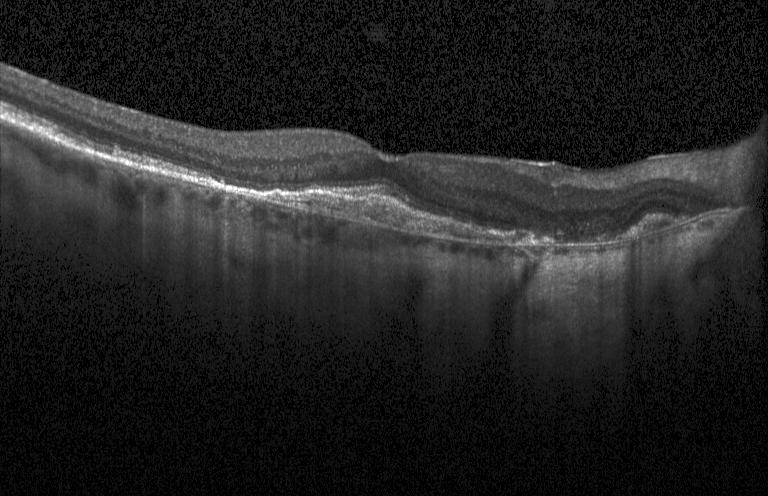

Spectral-domain optical coherence tomography, optical coherence tomography scan — The scan shows a choroidal neovascular membrane.